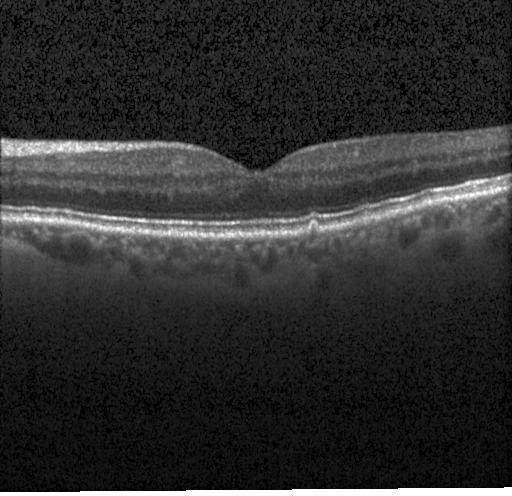
OCT B-scan, centered on the fovea, instrument: Heidelberg Spectralis
Diagnosis: multiple drusen.